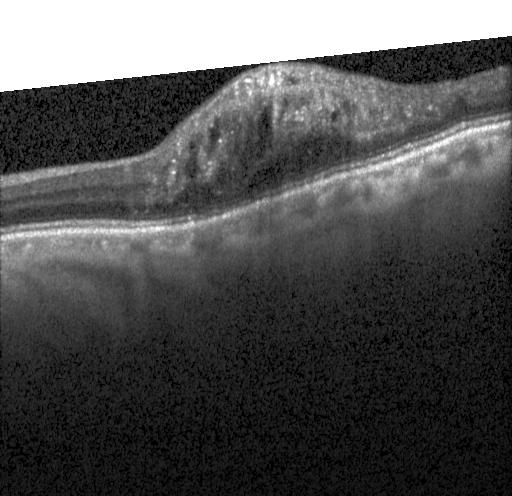

OCT B-scan
OCT finding: DME.